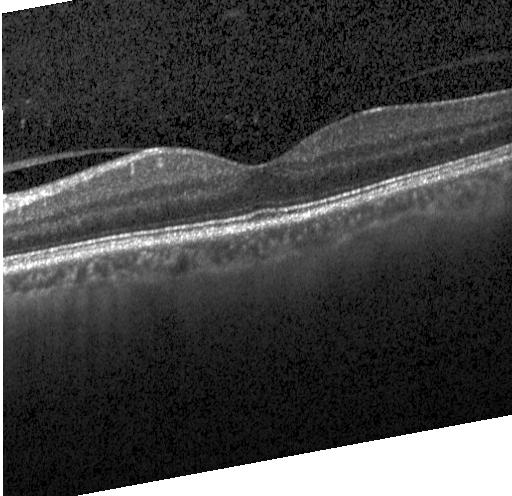
Optical coherence tomography scan. Impression: no choroidal neovascularization, diabetic macular edema, or drusen.